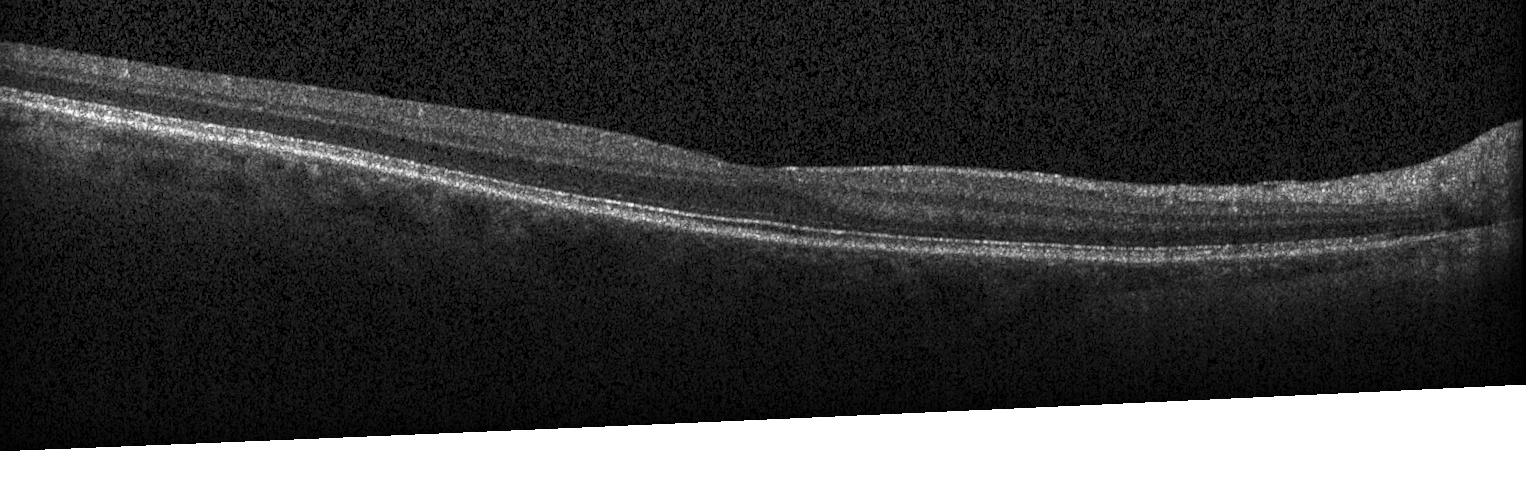

SD-OCT · macular scan · OCT line scan
No evidence of choroidal neovascularization, diabetic macular edema, or drusen.